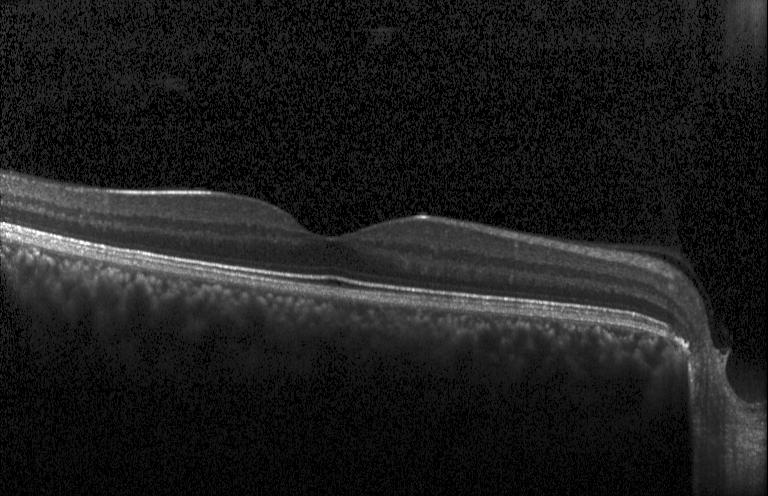

OCT B-scan. Instrument: Heidelberg Spectralis. Through the macula. Diagnosis: no choroidal neovascularization, no diabetic macular edema, and no drusen.